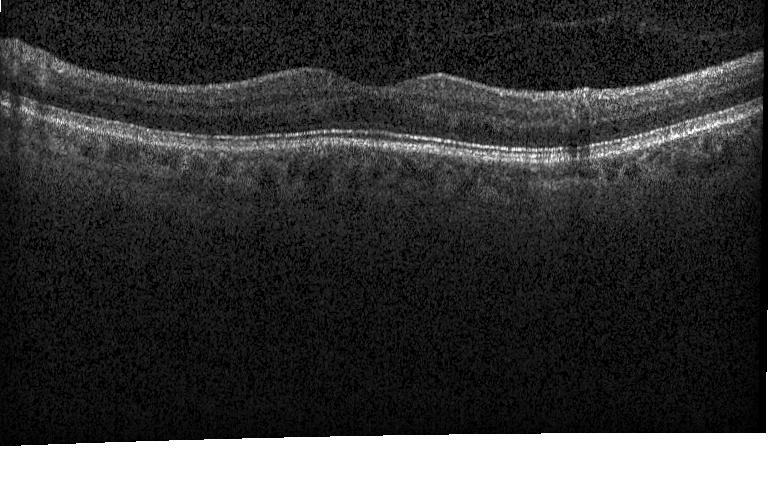

OCT B-scan
Dx: no choroidal neovascularization, no diabetic macular edema, and no drusen.